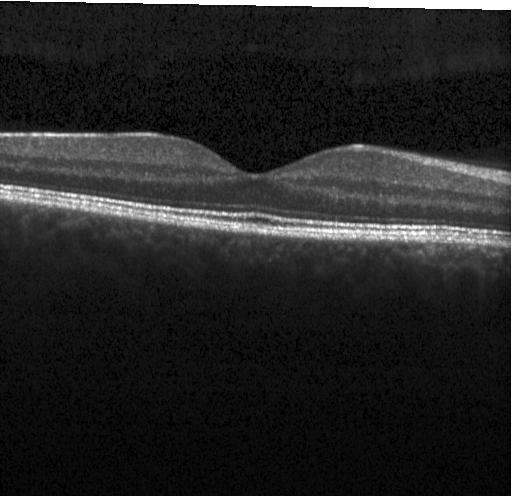 Optical coherence tomography scan; Heidelberg Spectralis; spectral-domain optical coherence tomography; macular scan
Finding: no CNV, no DME, and no drusen.